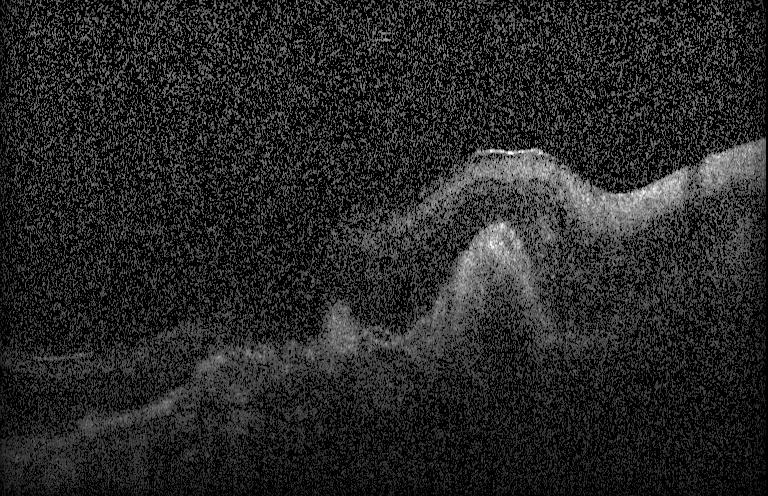
OCT B-scan — Macular OCT: a choroidal neovascular membrane.